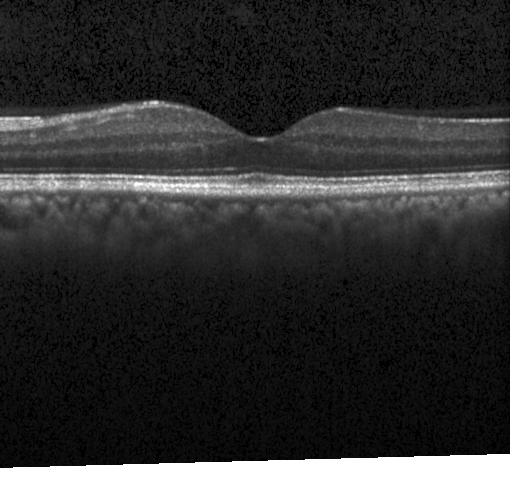 Retinal OCT cross-section; SD-OCT; centered on the fovea — Diagnosis: no choroidal neovascularization, diabetic macular edema, or drusen.